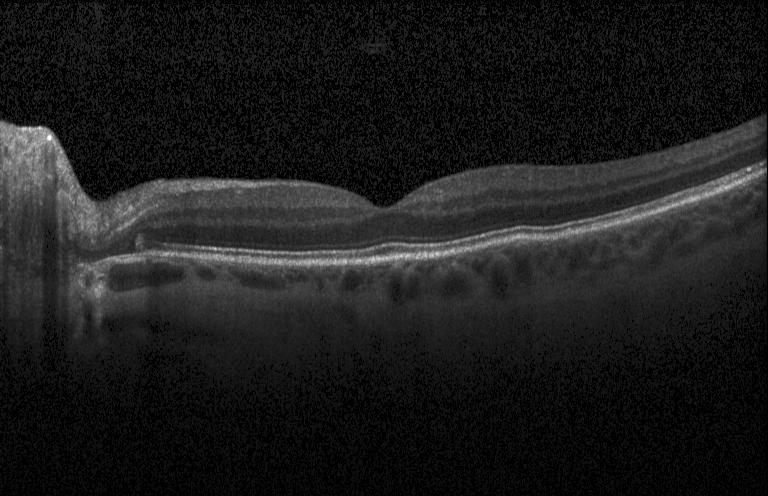

Optical coherence tomography scan. Assessment: neither choroidal neovascularization, diabetic macular edema, nor drusen.